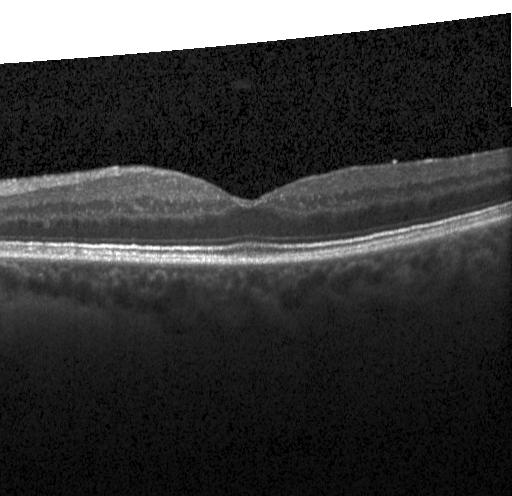 Spectral-domain optical coherence tomography, Heidelberg Spectralis OCT system, retinal OCT B-scan.
Diagnosis: no choroidal neovascularization, no diabetic macular edema, and no drusen.